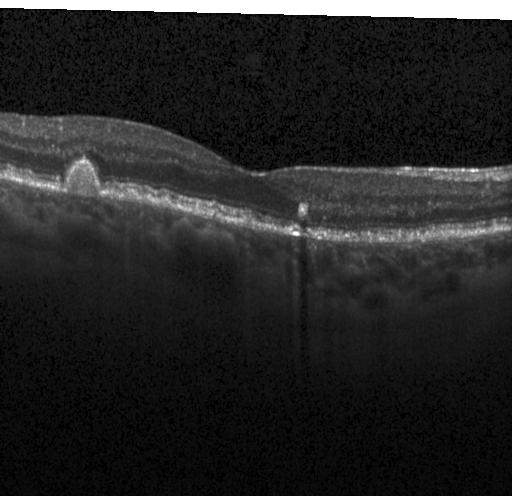

Spectral-domain OCT B-scan: drusen.